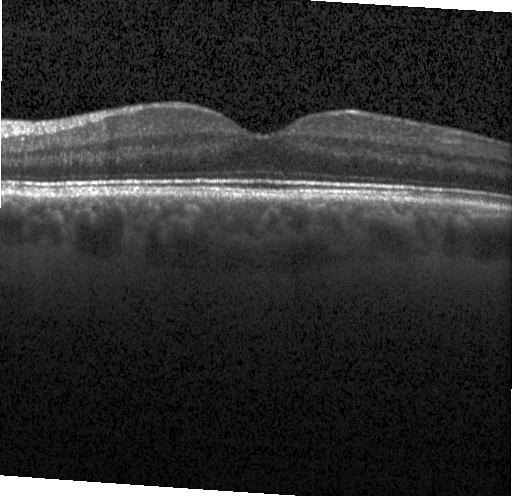
Retinal OCT cross-section.
This B-scan demonstrates no choroidal neovascularization, no diabetic macular edema, and no drusen.